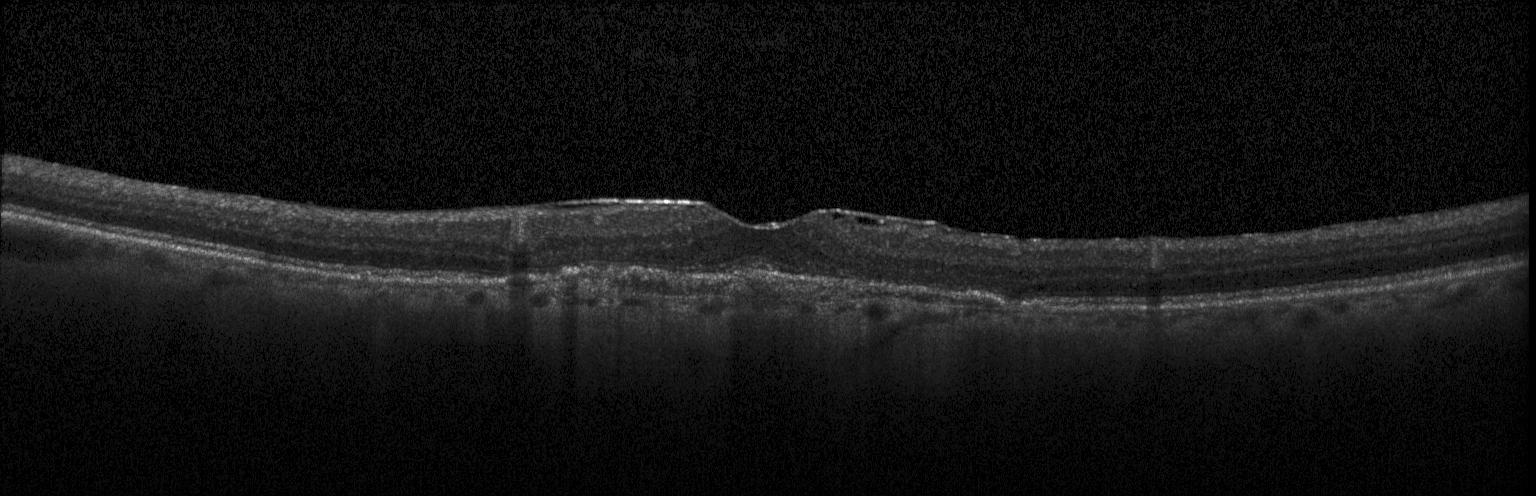 OCT line scan
Assessment: choroidal neovascularization (CNV).